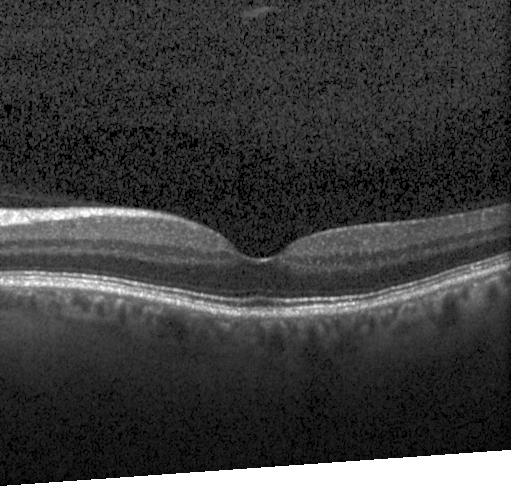
Retinal OCT cross-section showing neither CNV, DME, nor drusen.